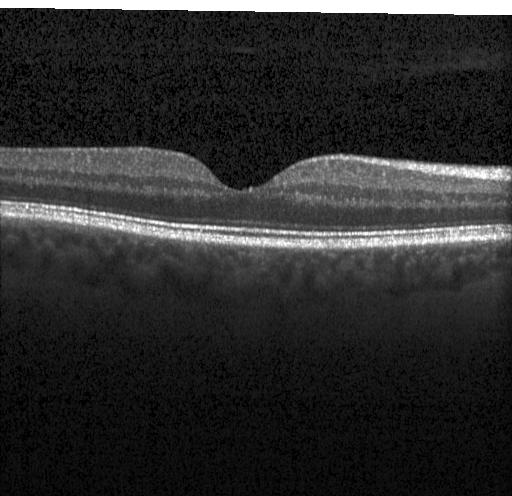 Optical coherence tomography B-scan
Macular OCT: neither choroidal neovascularization, diabetic macular edema, nor drusen.